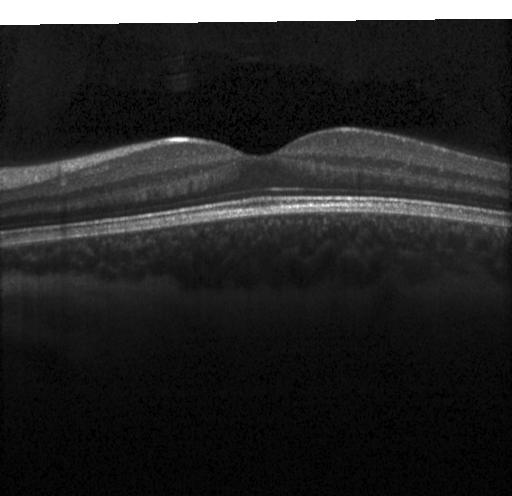

Horizontal scan through the fovea. Spectral-domain optical coherence tomography. Retinal OCT cross-section. Acquired on a Heidelberg Spectralis. Dx: no choroidal neovascularization, no diabetic macular edema, and no drusen.